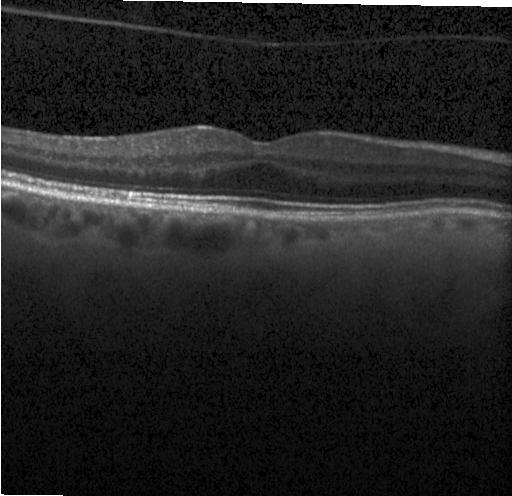 Heidelberg Spectralis, OCT B-scan
No evidence of CNV, DME, or drusen.